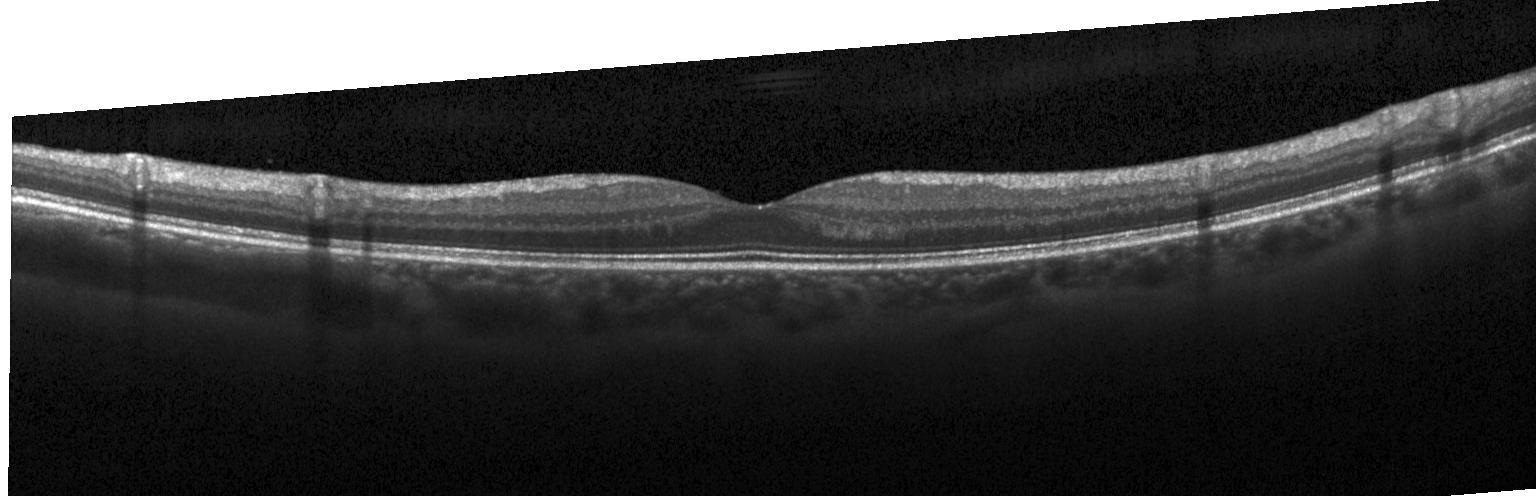 Retinal OCT cross-section; centered on the fovea; Heidelberg Spectralis OCT system — This B-scan demonstrates no choroidal neovascularization, diabetic macular edema, or drusen.